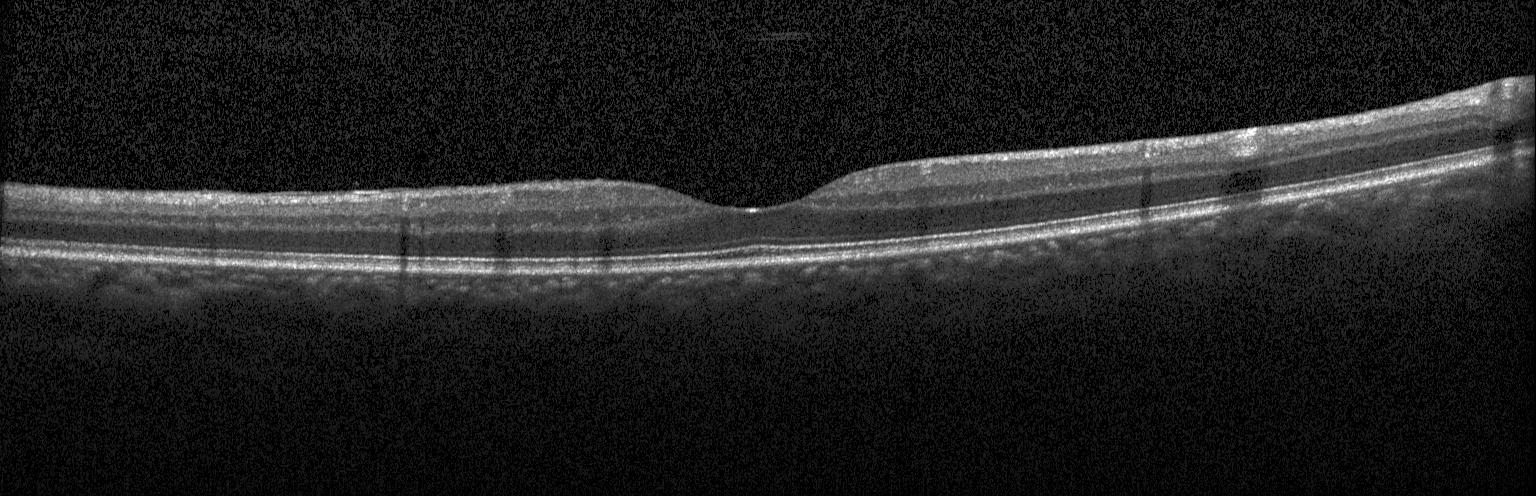

Retinal OCT B-scan · spectral-domain optical coherence tomography · Heidelberg Spectralis · centered on the fovea. Diagnosis: no choroidal neovascularization, diabetic macular edema, or drusen.